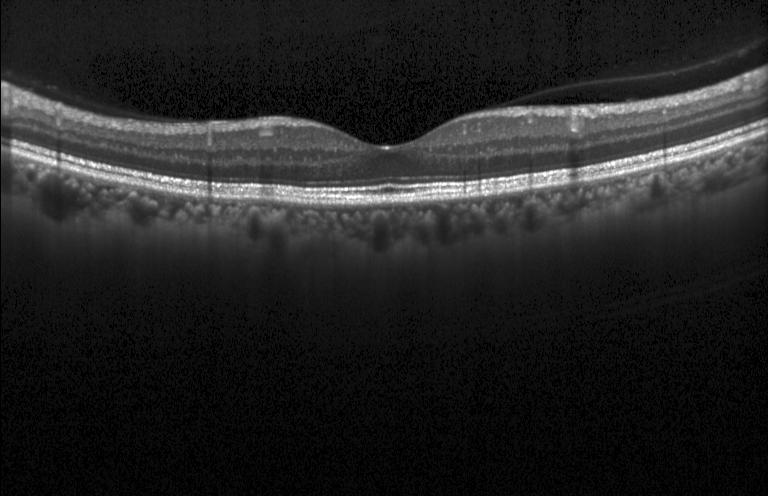

OCT finding: no evidence of choroidal neovascularization, diabetic macular edema, or drusen.